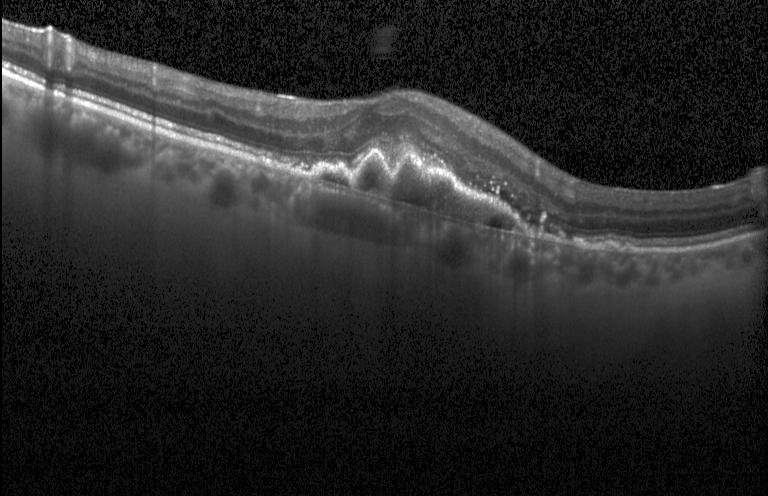
Fovea-centered · spectral-domain optical coherence tomography · OCT B-scan.
This B-scan demonstrates CNV.